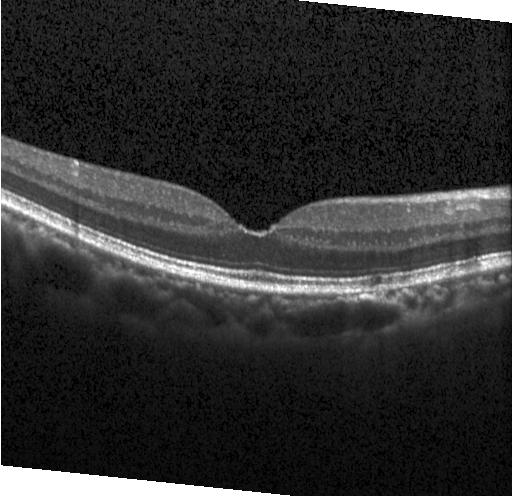

Diagnosis: no choroidal neovascularization, no diabetic macular edema, and no drusen.